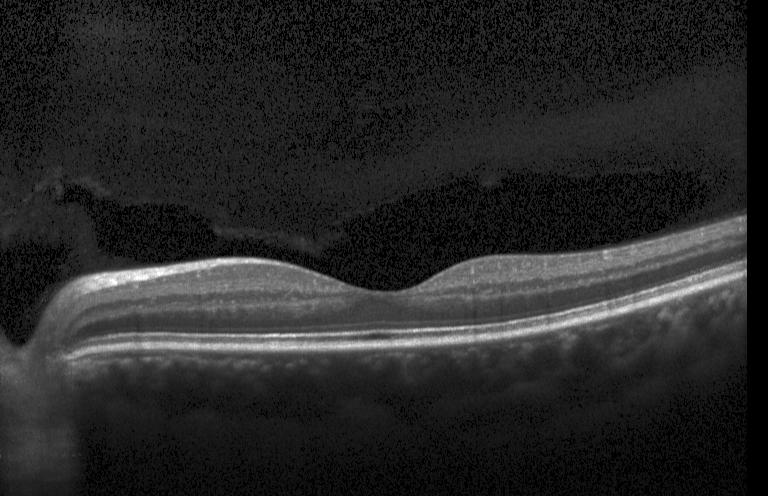

Optical coherence tomography B-scan. Centered on the fovea. Heidelberg Spectralis. Spectral-domain OCT — This B-scan demonstrates neither CNV, DME, nor drusen.